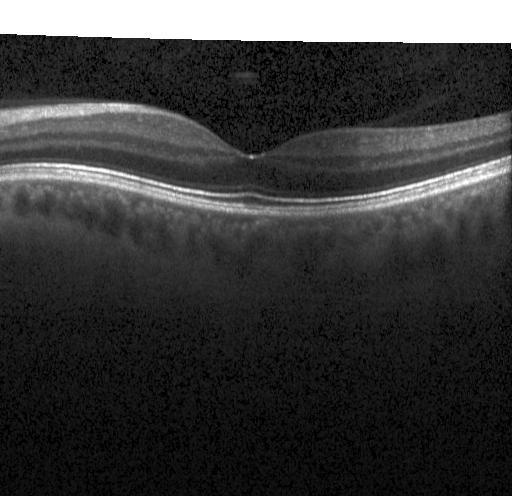

Finding: no choroidal neovascularization, no diabetic macular edema, and no drusen.